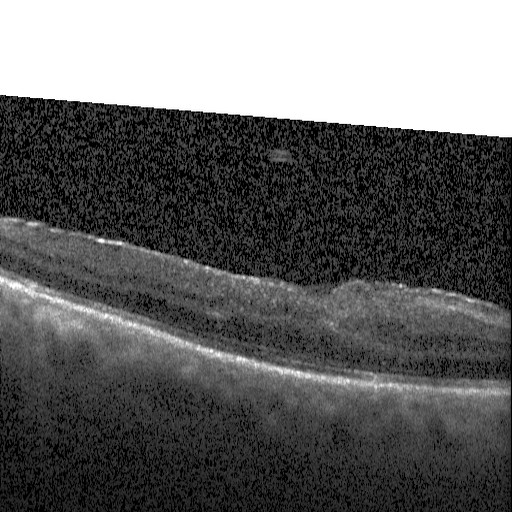
This B-scan demonstrates diabetic macular edema.